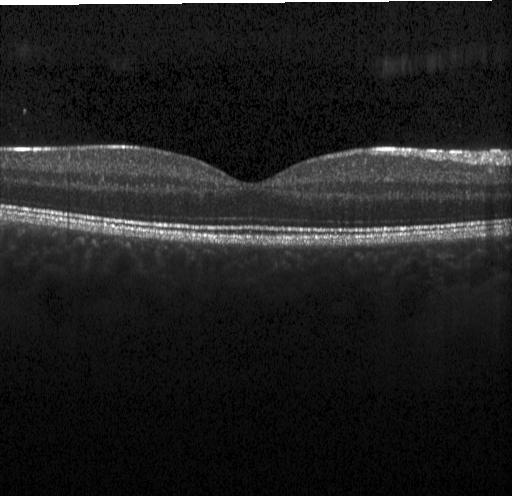

Heidelberg Spectralis; optical coherence tomography B-scan; spectral-domain optical coherence tomography. Finding: no CNV, no DME, and no drusen.